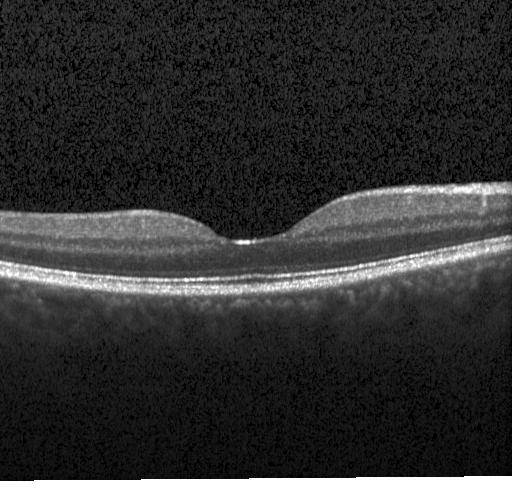
Optical coherence tomography B-scan
Assessment: neither choroidal neovascularization, diabetic macular edema, nor drusen.